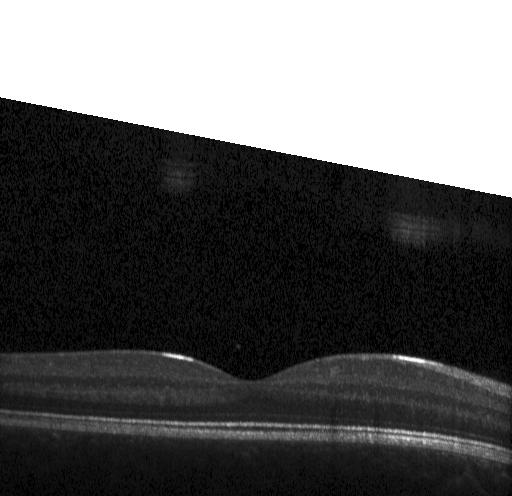 OCT B-scan.
Neither choroidal neovascularization, diabetic macular edema, nor drusen.